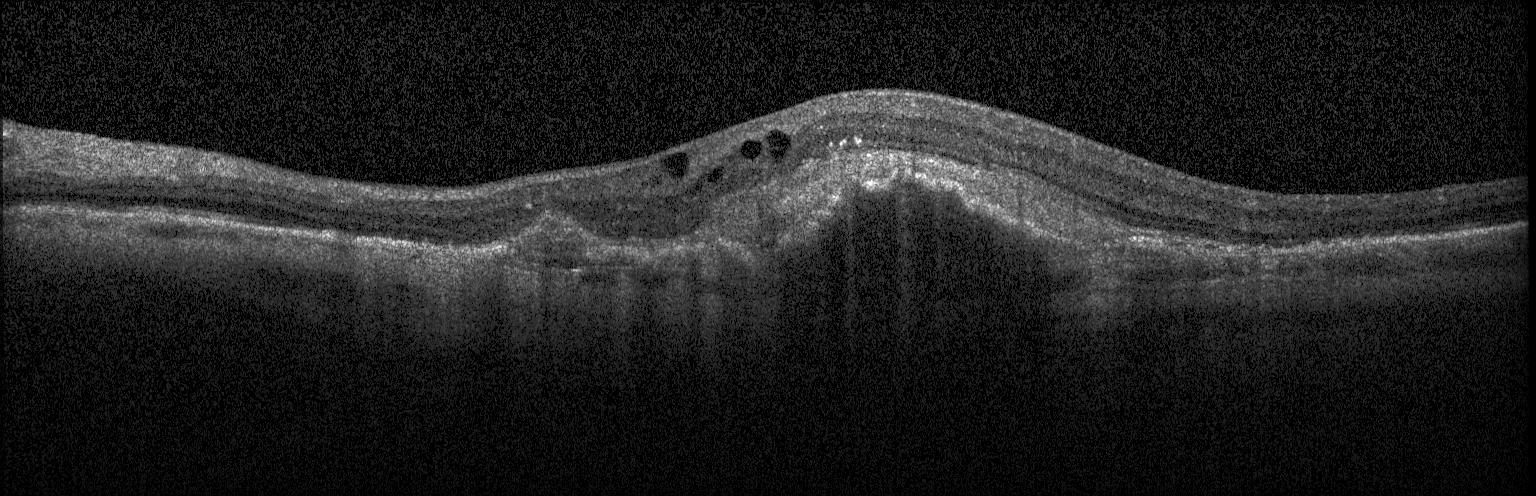

Through the macula. Spectral-domain optical coherence tomography. Optical coherence tomography scan.
Macular OCT: a choroidal neovascular membrane.